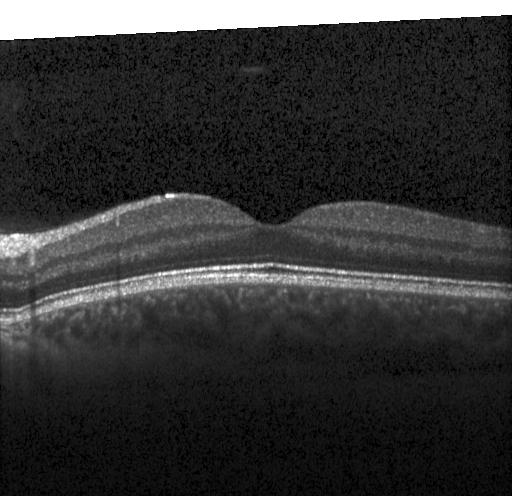 Centered on the fovea · OCT line scan · spectral-domain optical coherence tomography · instrument: Heidelberg Spectralis
Macular OCT: no evidence of CNV, DME, or drusen.